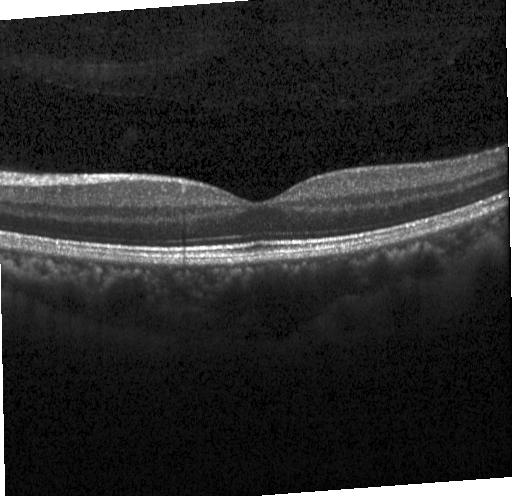 Horizontal scan through the fovea, retinal OCT B-scan, SD-OCT, instrument: Heidelberg Spectralis
Impression: no CNV, DME, or drusen.